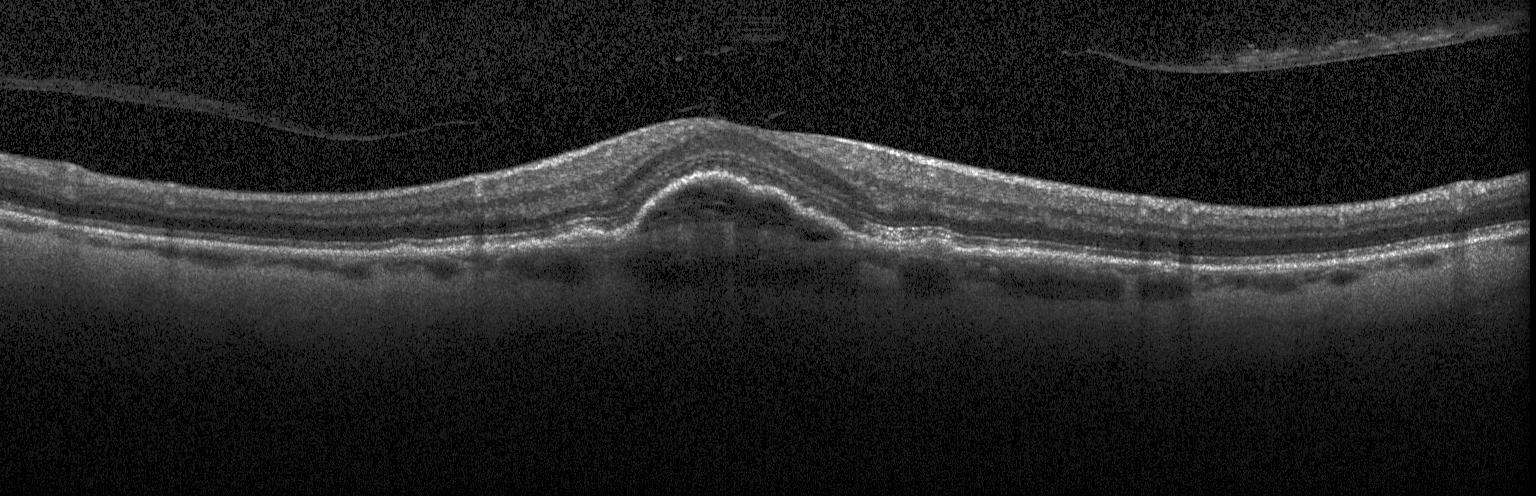

Fovea-centered. Retinal OCT cross-section.
Macular OCT: a choroidal neovascular membrane.